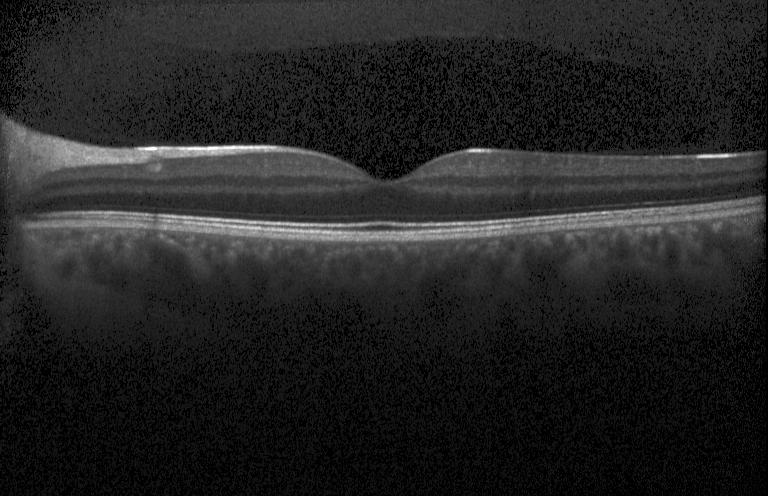

SD-OCT · OCT B-scan · acquired on a Heidelberg Spectralis. Finding: no choroidal neovascularization, no diabetic macular edema, and no drusen.